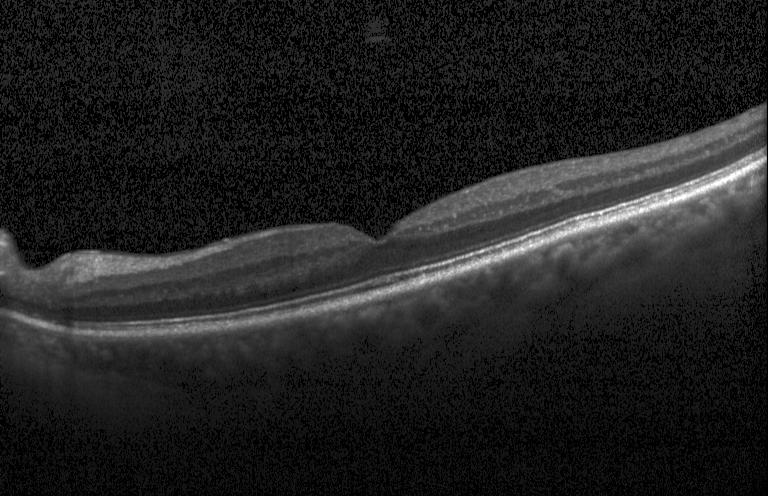 Finding: no choroidal neovascularization, diabetic macular edema, or drusen.